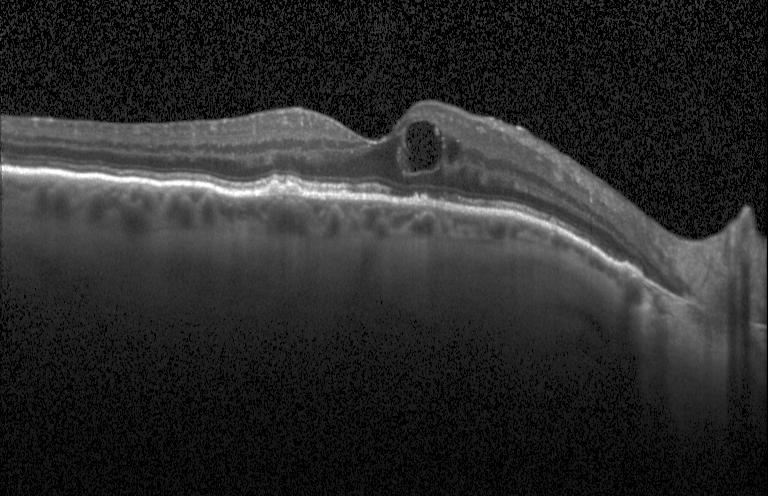
Impression: choroidal neovascularization (CNV).